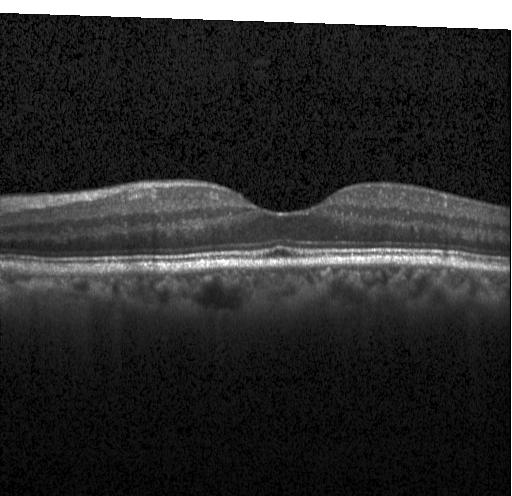
Impression: no CNV, DME, or drusen.